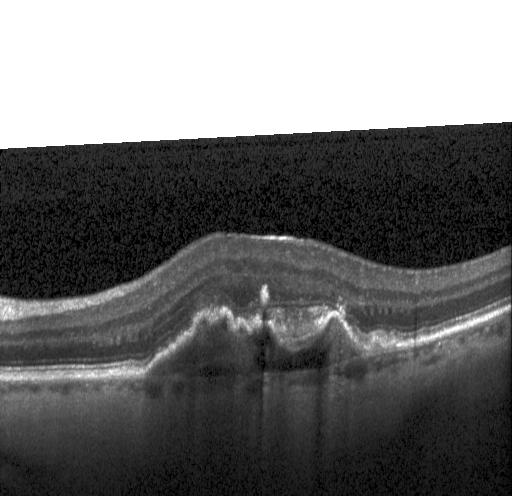

Macular scan. Optical coherence tomography scan. SD-OCT. Instrument: Heidelberg Spectralis
A choroidal neovascular membrane.